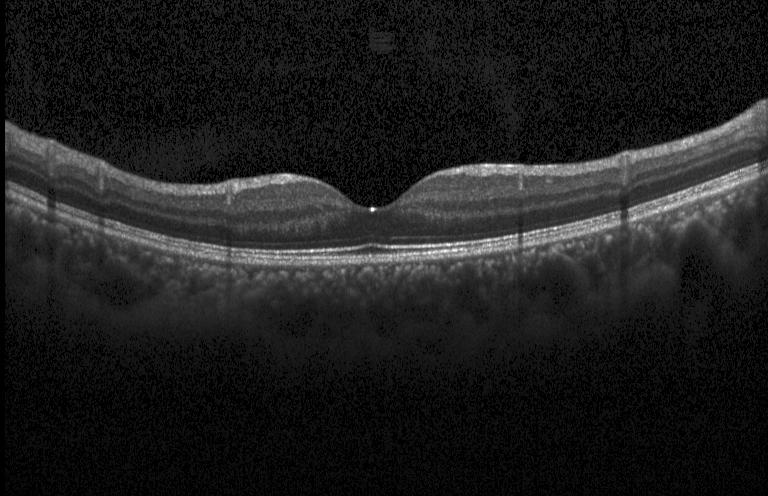
Spectral-domain OCT · Heidelberg Spectralis OCT system · horizontal scan through the fovea · OCT line scan — Macular OCT: no CNV, DME, or drusen.